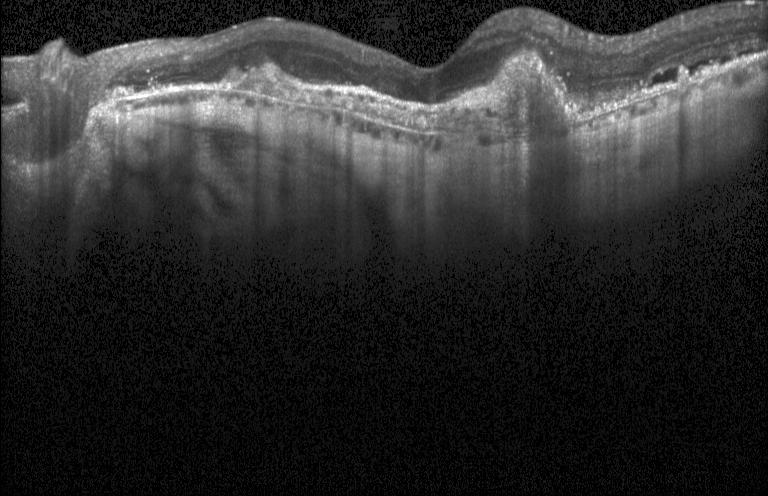
Centered on the fovea. OCT line scan.
Diagnosis: a choroidal neovascular membrane.